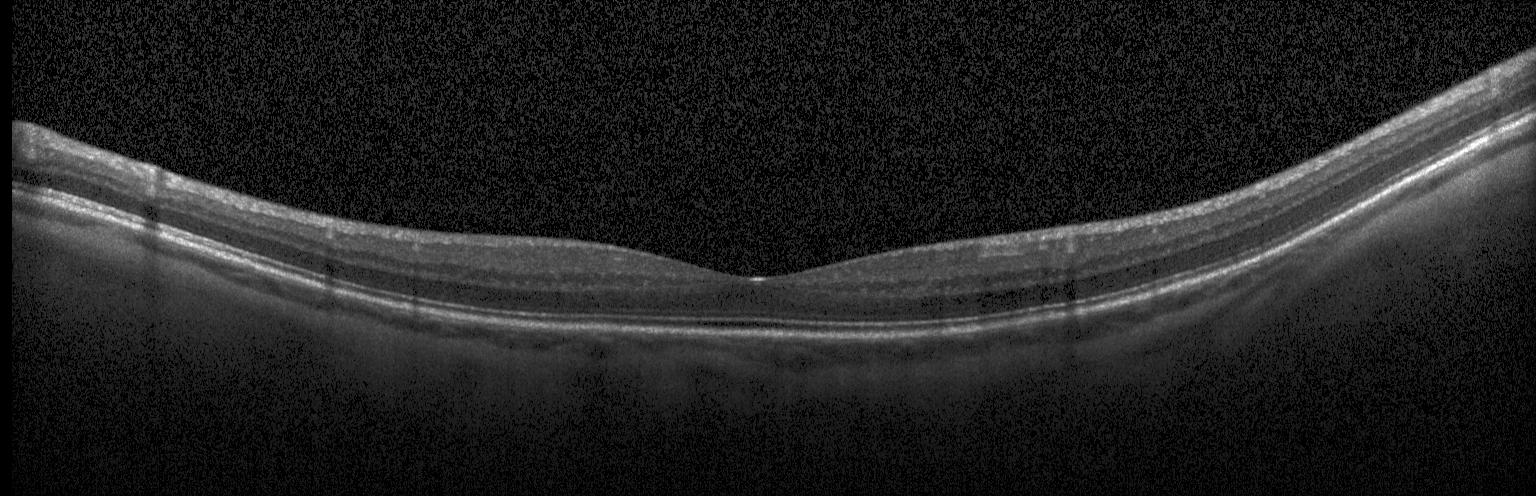

Macular scan, acquired on a Heidelberg Spectralis, OCT line scan. Diagnosis: neither choroidal neovascularization, diabetic macular edema, nor drusen.